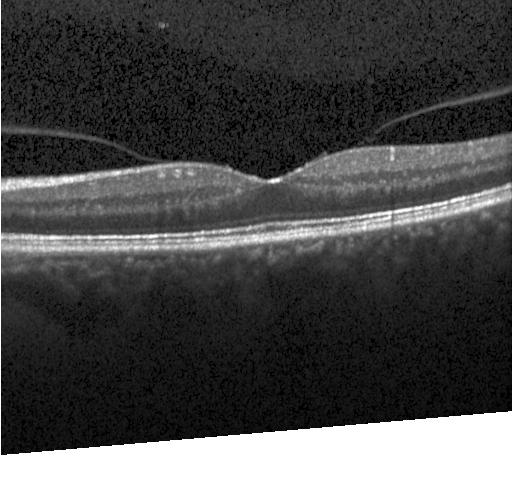
Impression: neither choroidal neovascularization, diabetic macular edema, nor drusen.